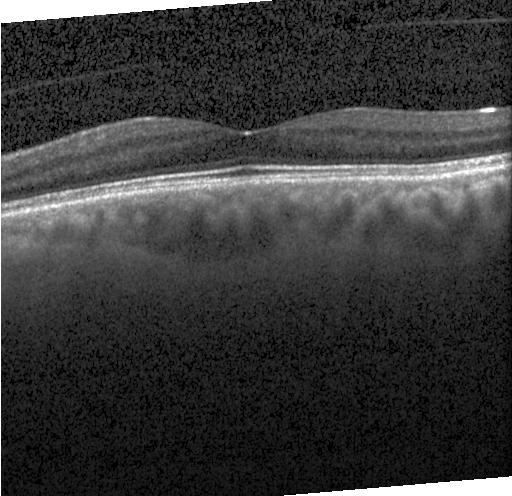

Dx: no evidence of CNV, DME, or drusen.